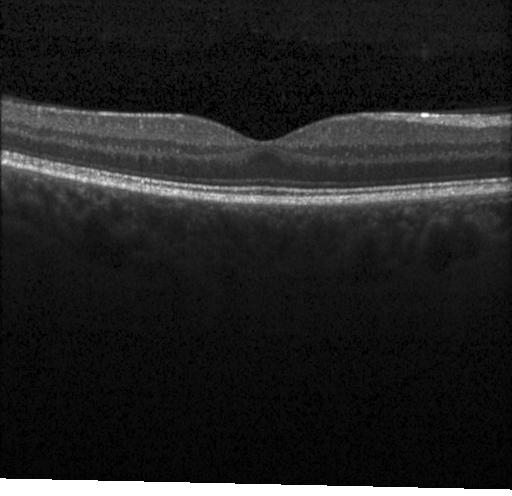

Retinal OCT cross-section. Assessment: no evidence of choroidal neovascularization, diabetic macular edema, or drusen.